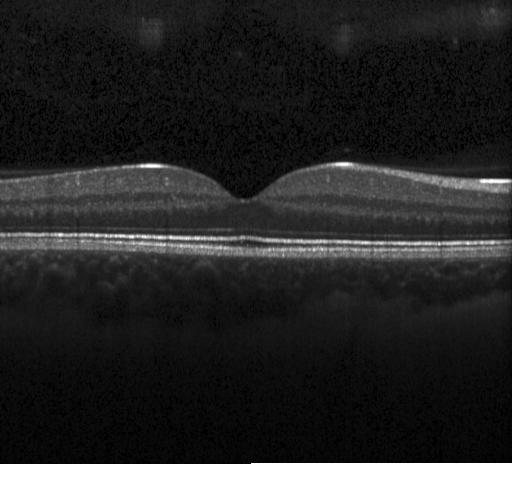
Optical coherence tomography scan, Heidelberg Spectralis OCT system, SD-OCT, fovea-centered. Neither CNV, DME, nor drusen.